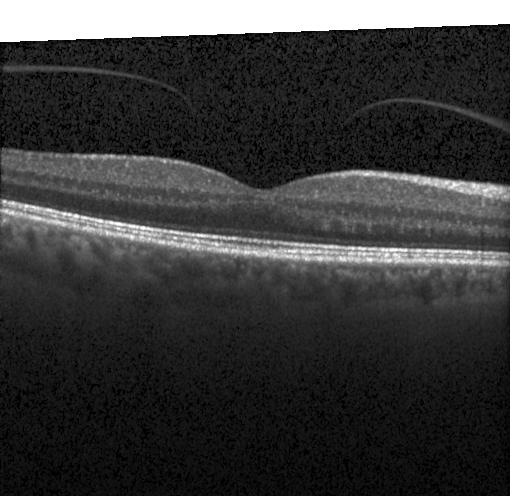
Macular OCT demonstrating no evidence of CNV, DME, or drusen.